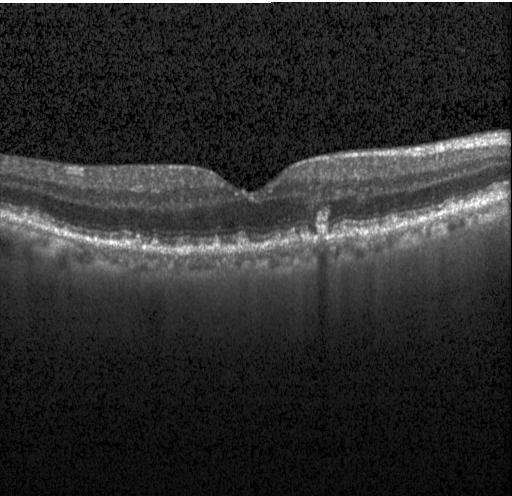 Spectral-domain optical coherence tomography, retinal OCT cross-section, horizontal scan through the fovea. This B-scan demonstrates drusen.